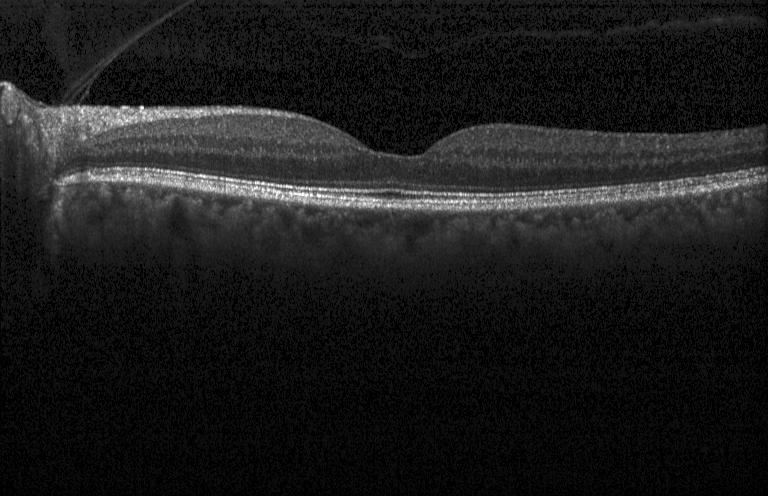 Diagnosis: no choroidal neovascularization, no diabetic macular edema, and no drusen.